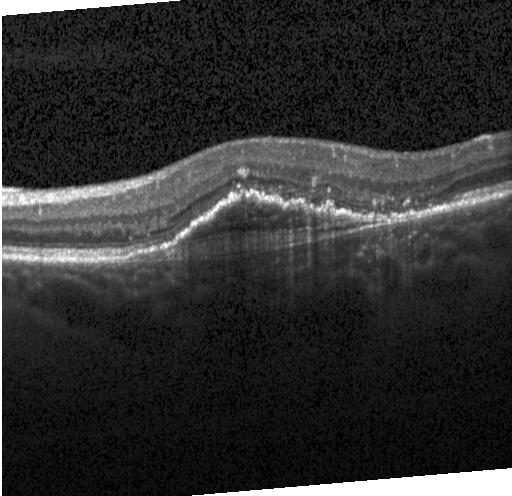
Assessment: a choroidal neovascular membrane.